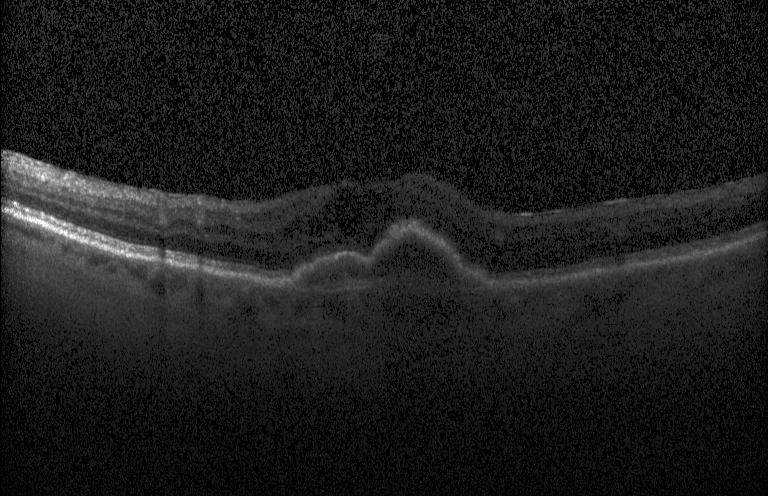
OCT line scan. Fovea-centered. Spectral-domain optical coherence tomography. Impression: choroidal neovascularization (CNV).